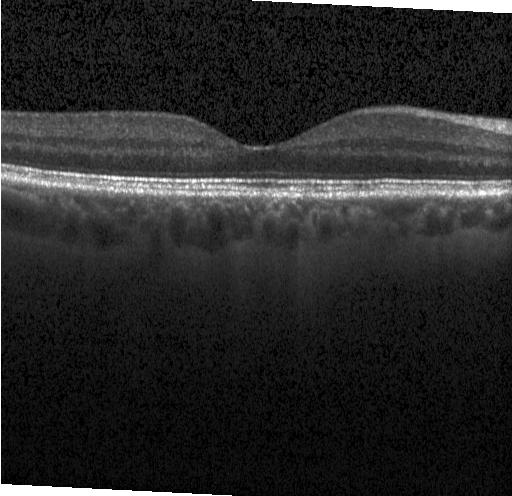
Spectral-domain OCT B-scan: neither choroidal neovascularization, diabetic macular edema, nor drusen.